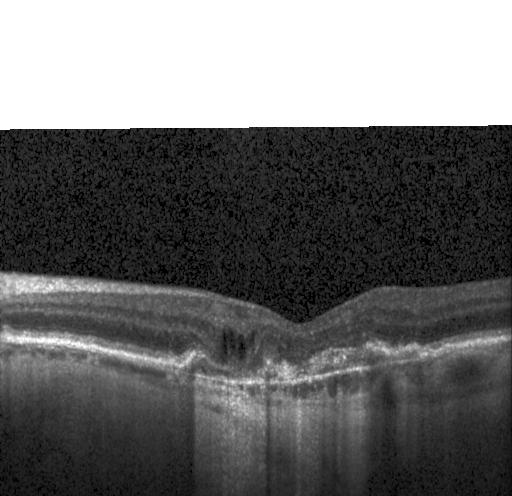
Through the macula, OCT line scan — Impression: CNV.